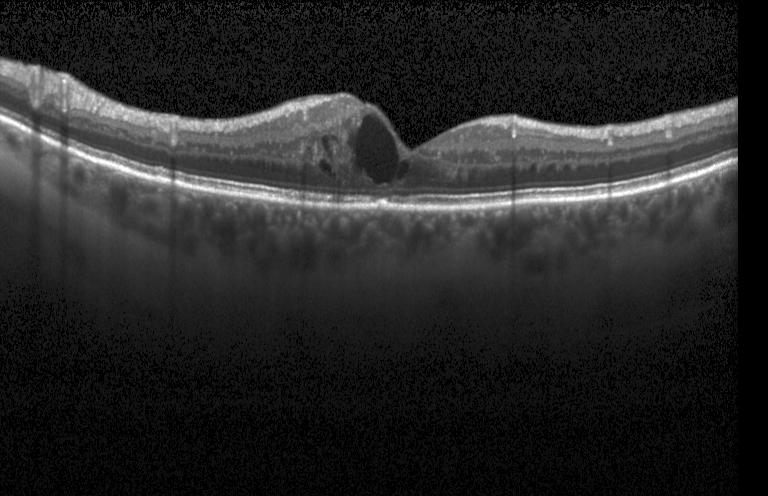 Finding: DME.